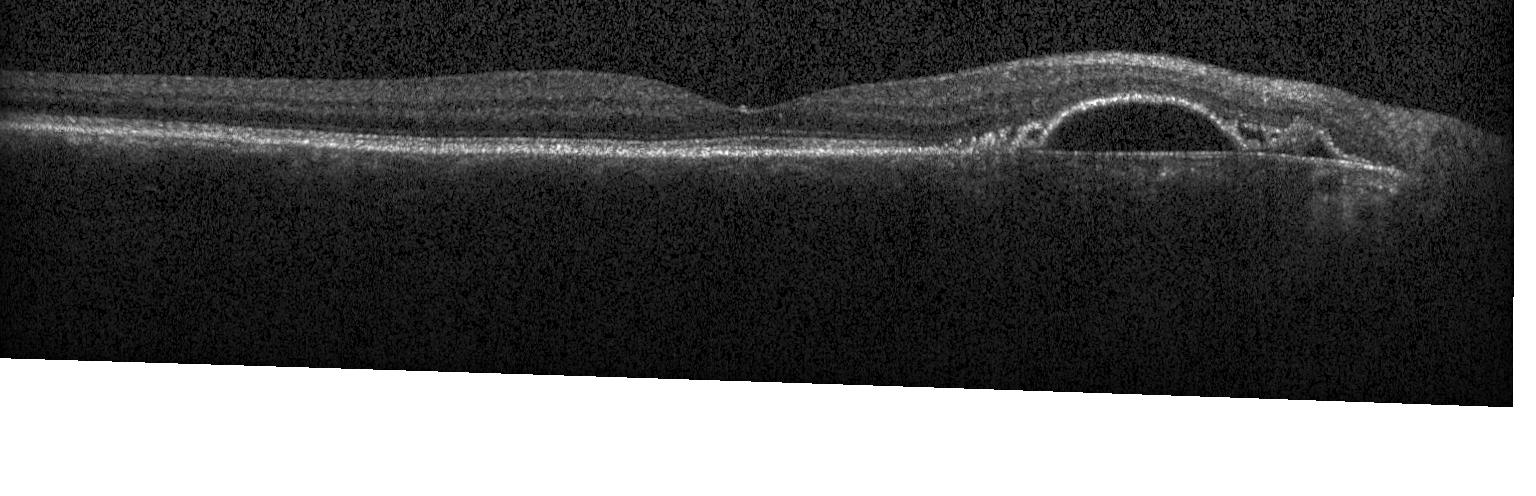
Impression: a choroidal neovascular membrane.